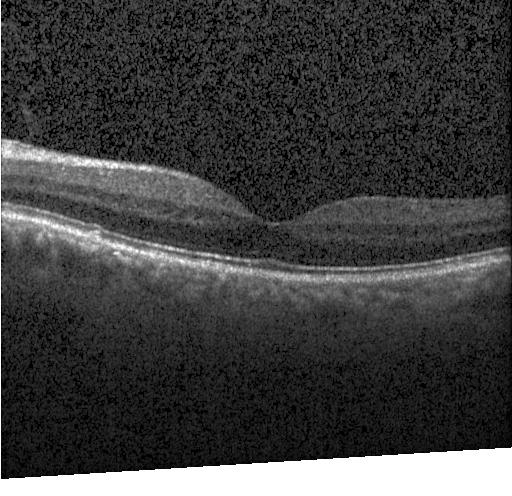 OCT scan showing sub-RPE drusenoid deposits.